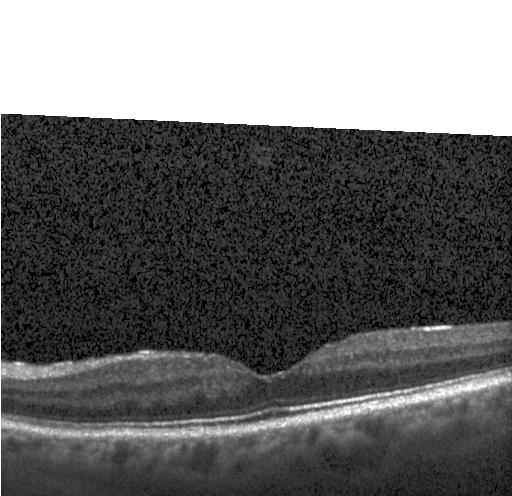 Macular OCT: no CNV, no DME, and no drusen.